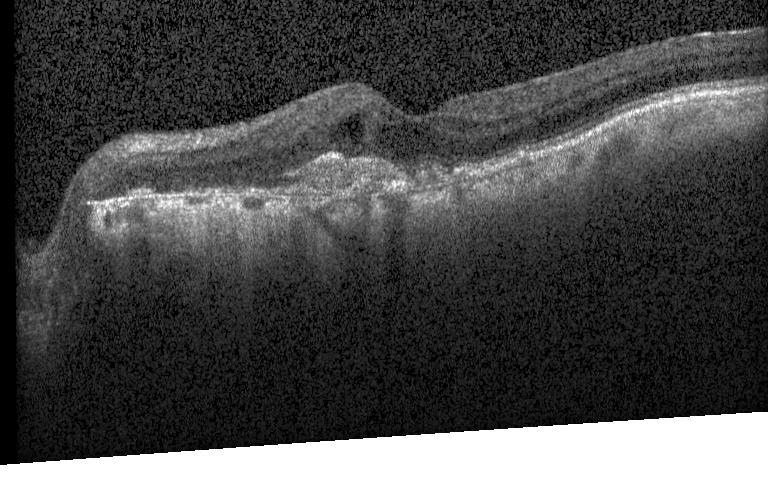 Retinal OCT B-scan.
This B-scan demonstrates a choroidal neovascular membrane.